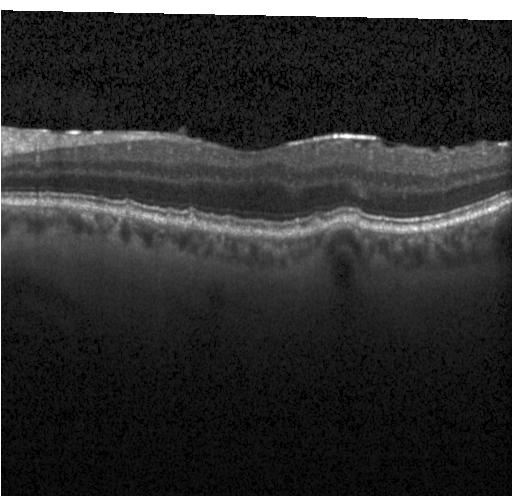

This B-scan demonstrates sub-RPE drusenoid deposits.